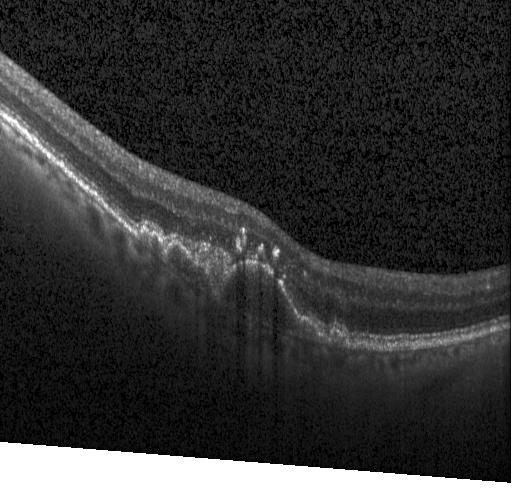
Finding: choroidal neovascularization.